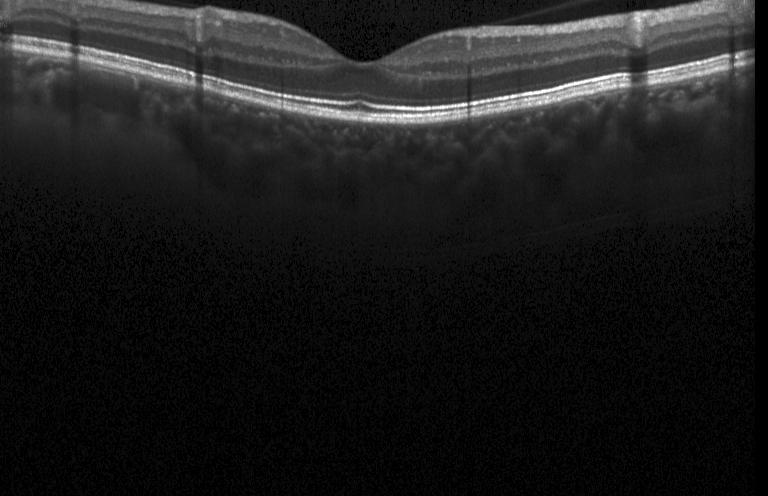

OCT B-scan; centered on the fovea; acquired on a Heidelberg Spectralis — Finding: no CNV, DME, or drusen.